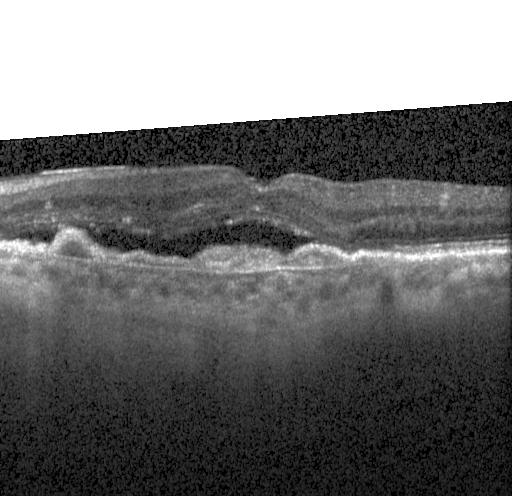 Retinal OCT cross-section.
Impression: choroidal neovascularization (CNV).